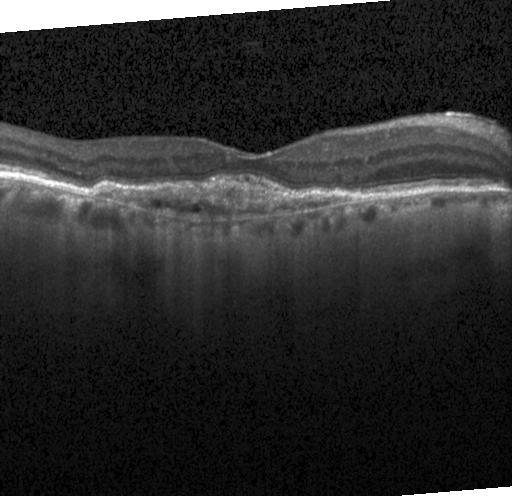
Acquired on a Heidelberg Spectralis, retinal OCT cross-section. Finding: a choroidal neovascular membrane.